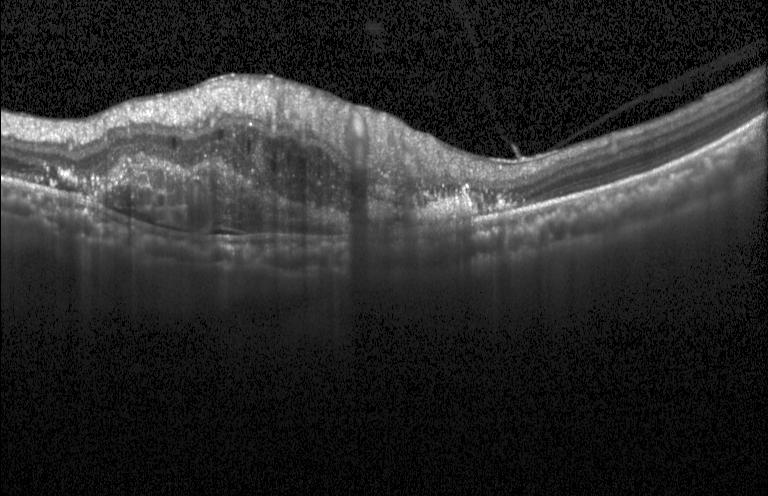 Retinal OCT B-scan, Heidelberg Spectralis, through the macula, spectral-domain optical coherence tomography. Impression: CNV.